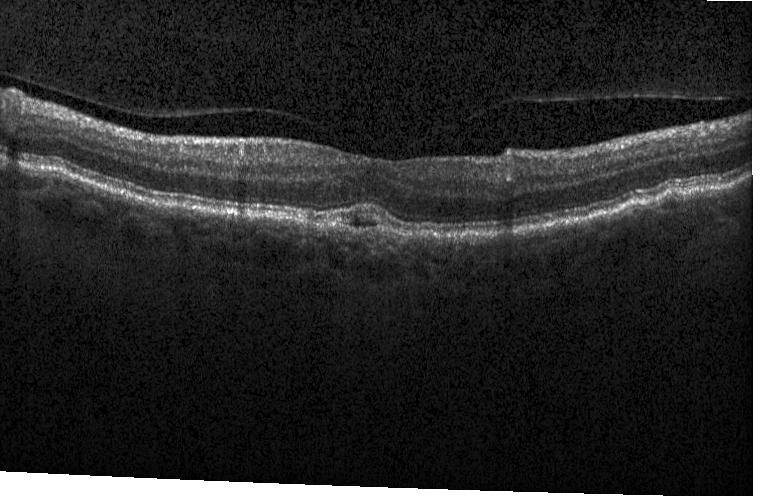

OCT line scan · macular scan.
Finding: a choroidal neovascular membrane.